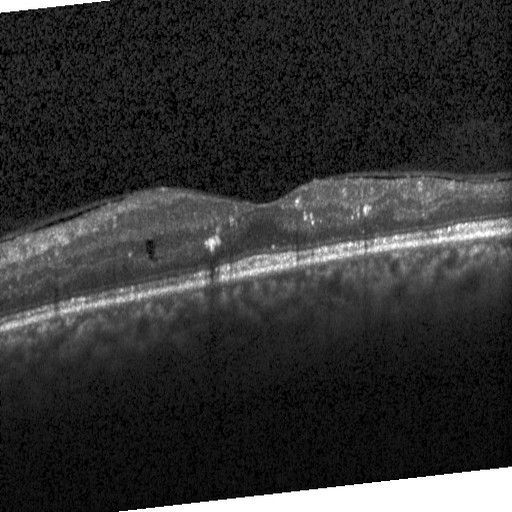
OCT finding: DME.